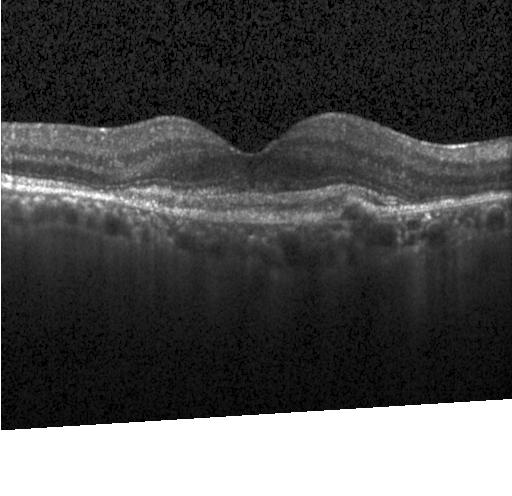

Retinal OCT cross-section.
The scan shows CNV.